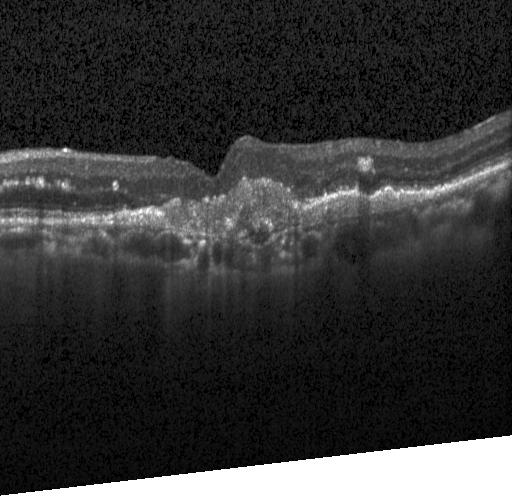 OCT finding: a choroidal neovascular membrane.